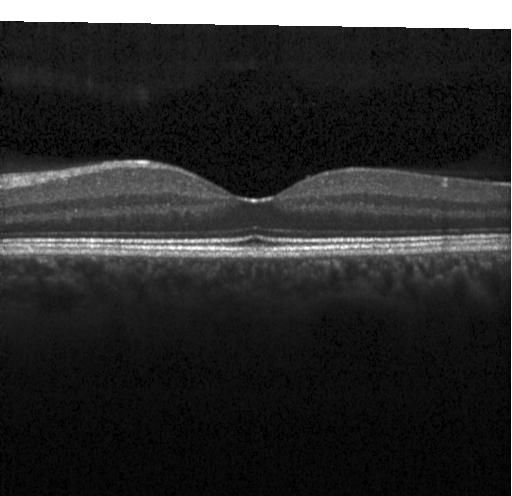
This B-scan demonstrates neither CNV, DME, nor drusen.